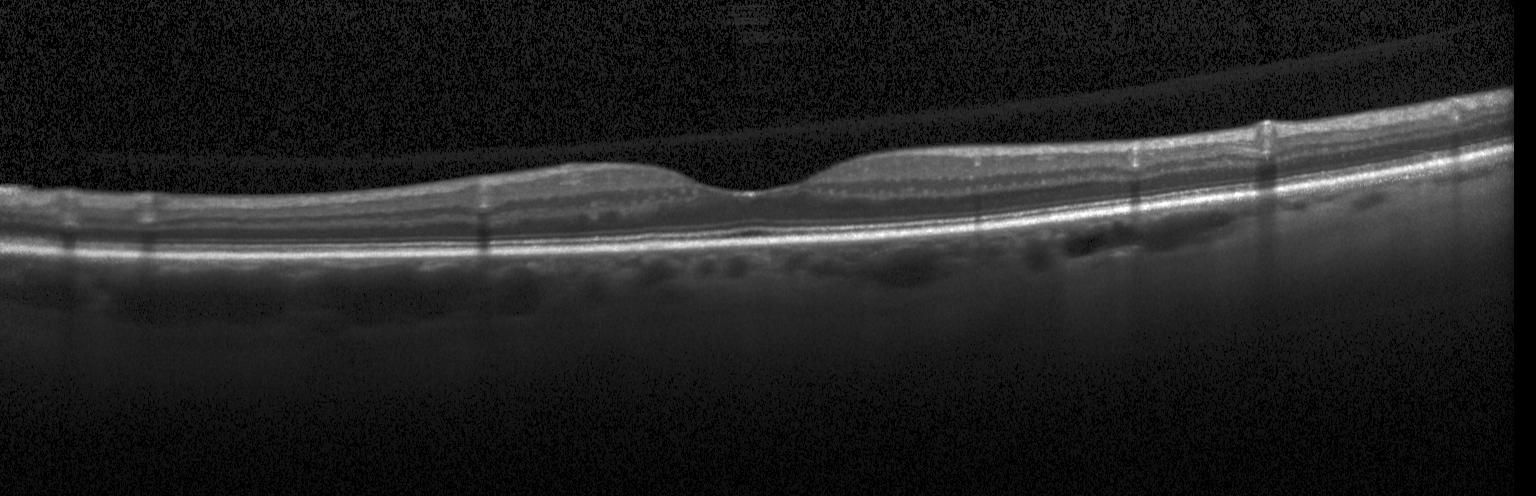

OCT line scan; centered on the fovea; SD-OCT. The scan shows neither choroidal neovascularization, diabetic macular edema, nor drusen.